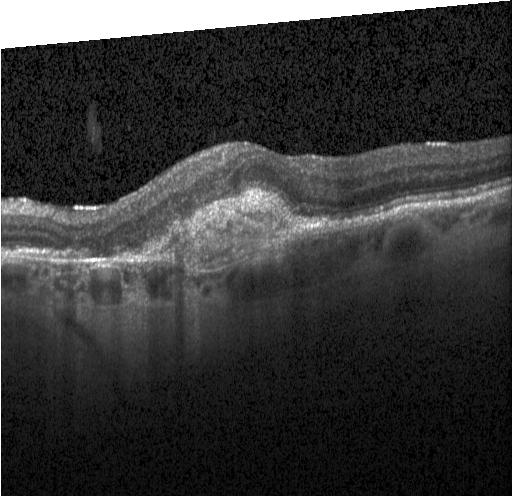
Assessment: choroidal neovascularization.